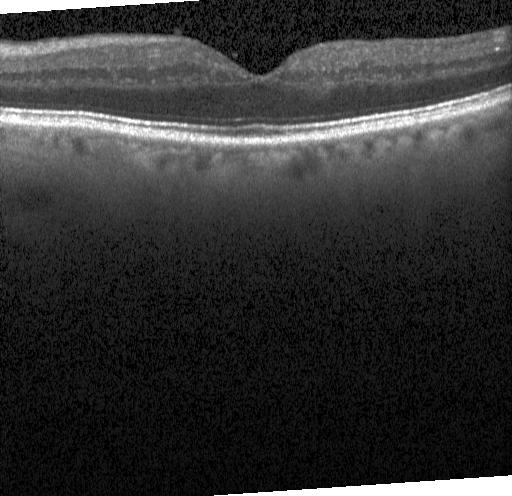 Retinal OCT cross-section showing no choroidal neovascularization, diabetic macular edema, or drusen.